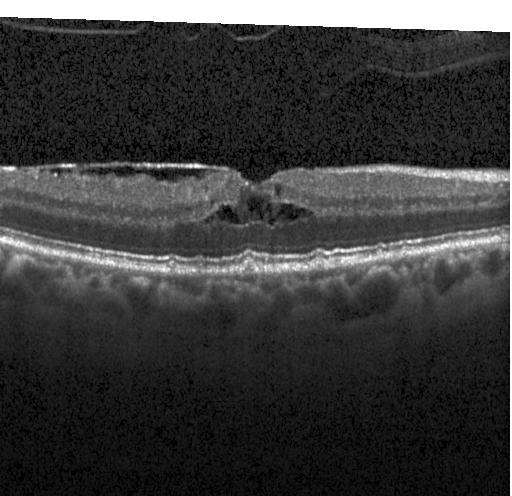 Drusen.